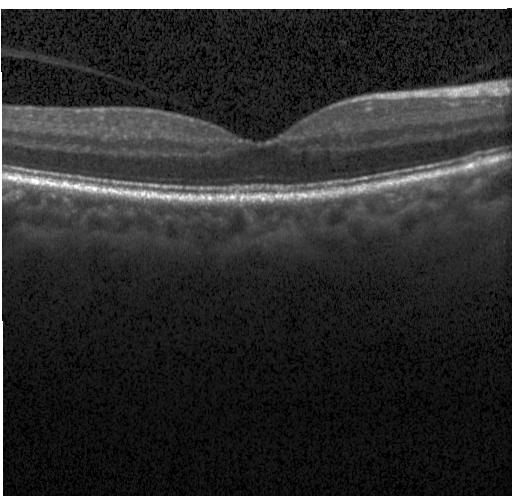
Impression: neither choroidal neovascularization, diabetic macular edema, nor drusen.